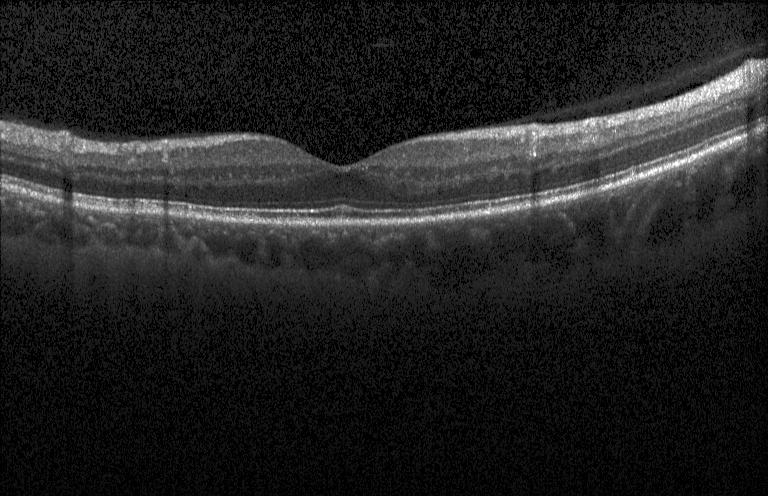 OCT finding: no choroidal neovascularization, no diabetic macular edema, and no drusen.